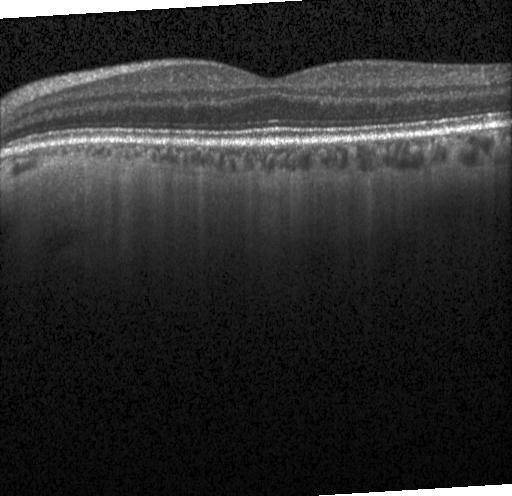 OCT scan showing no choroidal neovascularization, no diabetic macular edema, and no drusen.